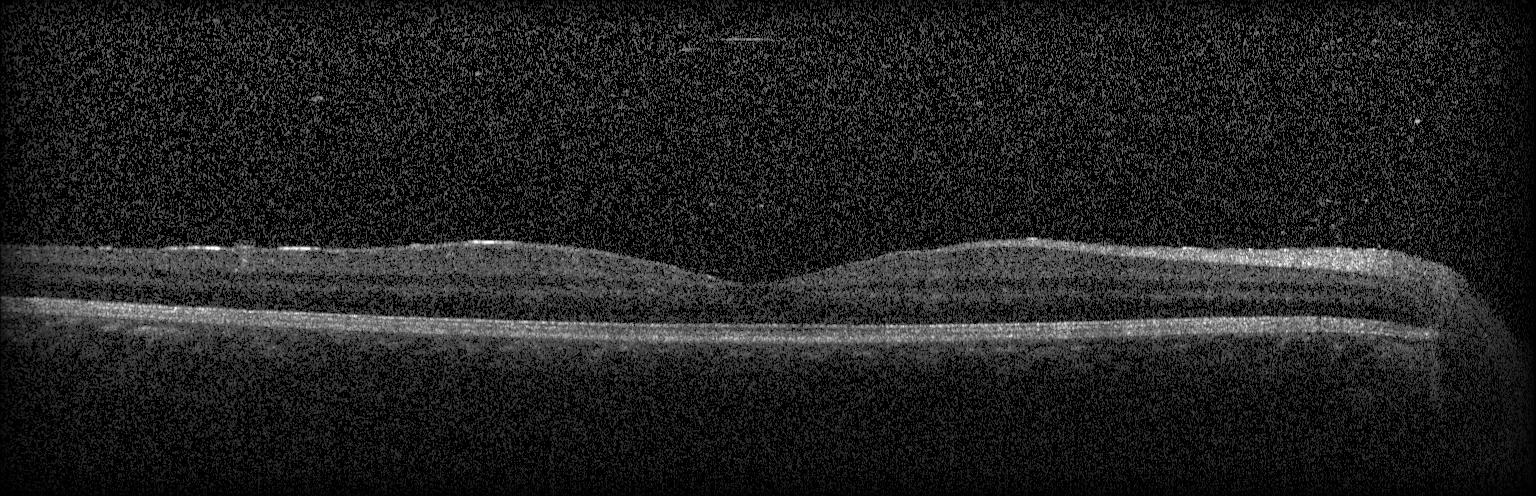
Dx: no choroidal neovascularization, diabetic macular edema, or drusen.